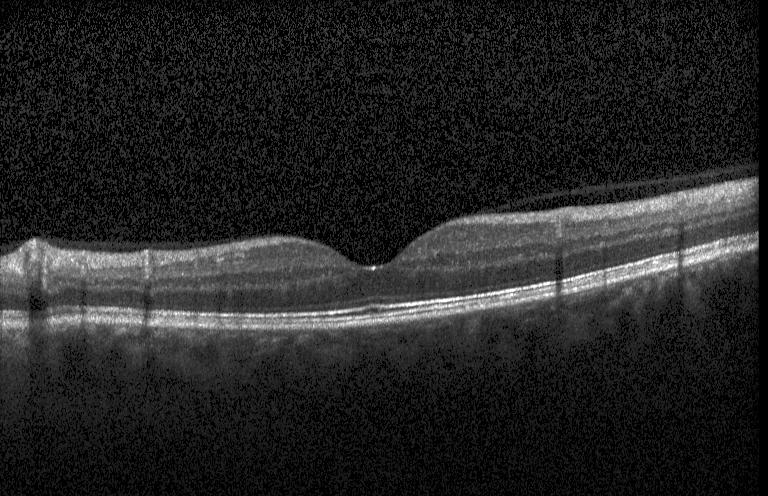
Optical coherence tomography B-scan
Macular OCT: neither choroidal neovascularization, diabetic macular edema, nor drusen.